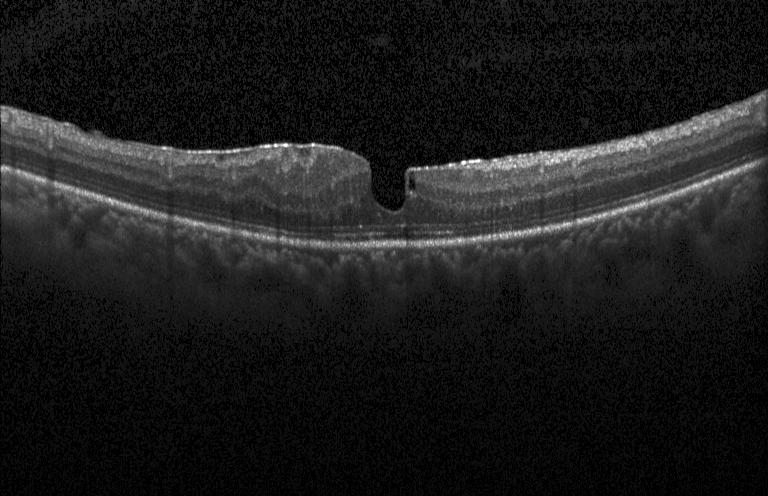

Acquired on a Heidelberg Spectralis; horizontal scan through the fovea; SD-OCT; optical coherence tomography scan.
The scan shows diabetic macular edema (DME).